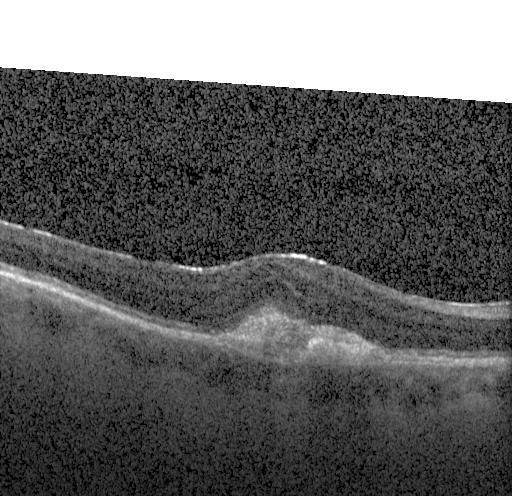

Instrument: Heidelberg Spectralis, retinal OCT B-scan, horizontal scan through the fovea, SD-OCT.
CNV.